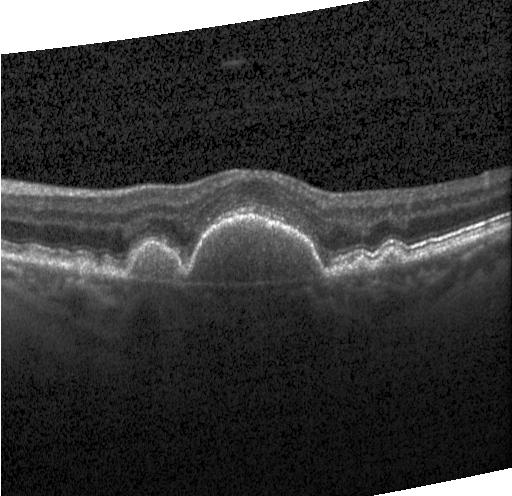
OCT line scan. Acquired on a Heidelberg Spectralis — Finding: a choroidal neovascular membrane.